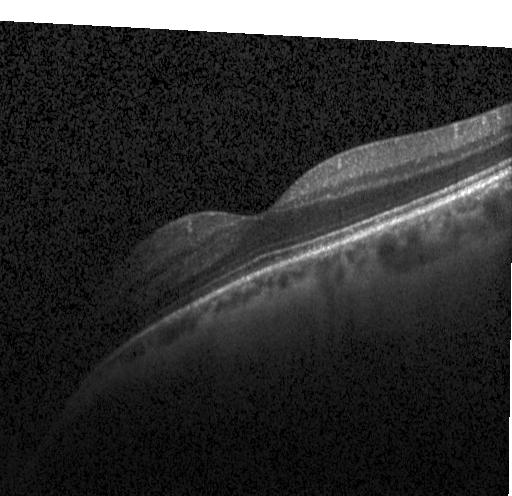
Spectral-domain OCT B-scan: neither choroidal neovascularization, diabetic macular edema, nor drusen.